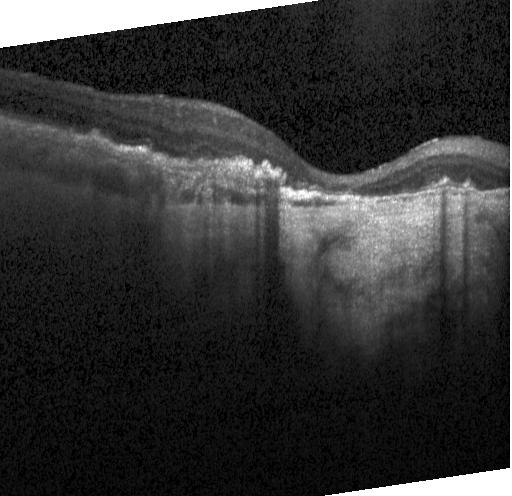

Dx: choroidal neovascularization.